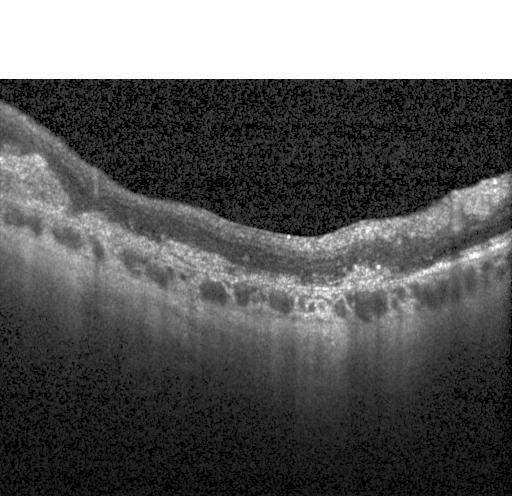

Optical coherence tomography scan; SD-OCT; instrument: Heidelberg Spectralis.
Dx: a choroidal neovascular membrane.